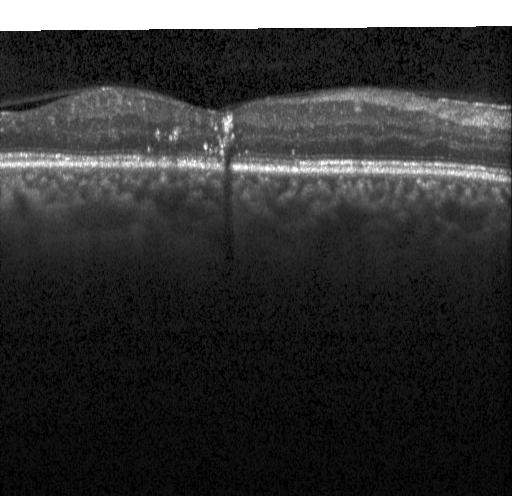 Finding: diabetic macular edema.